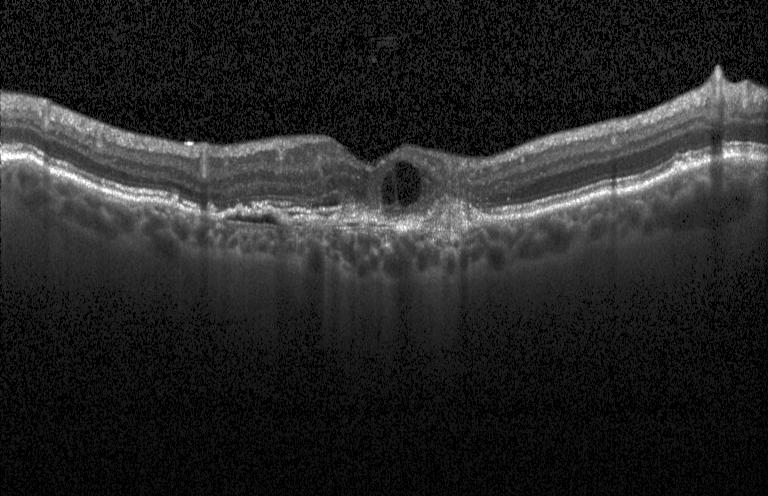

Instrument: Heidelberg Spectralis, retinal OCT B-scan — Assessment: choroidal neovascularization.